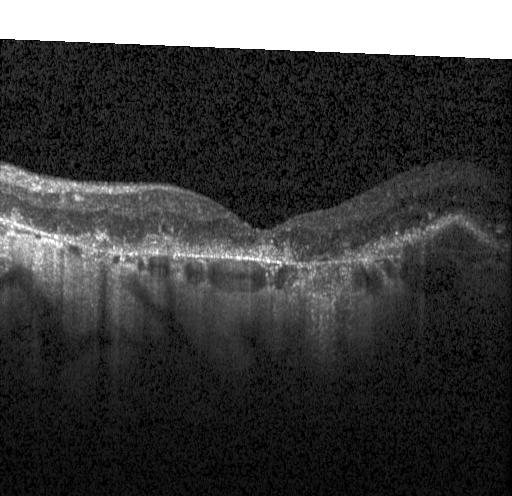 Spectral-domain OCT B-scan: choroidal neovascularization (CNV).